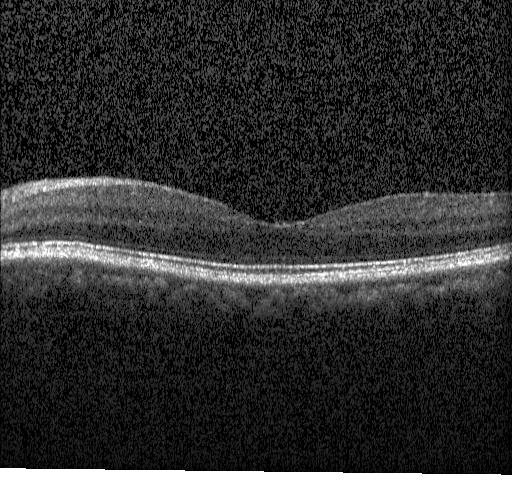

Optical coherence tomography B-scan · SD-OCT. Dx: neither choroidal neovascularization, diabetic macular edema, nor drusen.